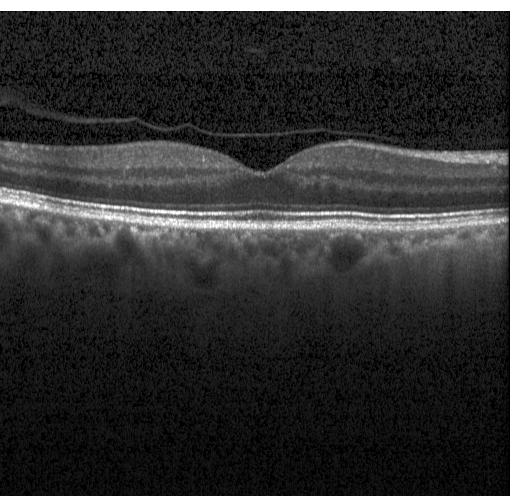 Heidelberg Spectralis; SD-OCT; macular scan; retinal OCT cross-section.
Impression: no CNV, no DME, and no drusen.